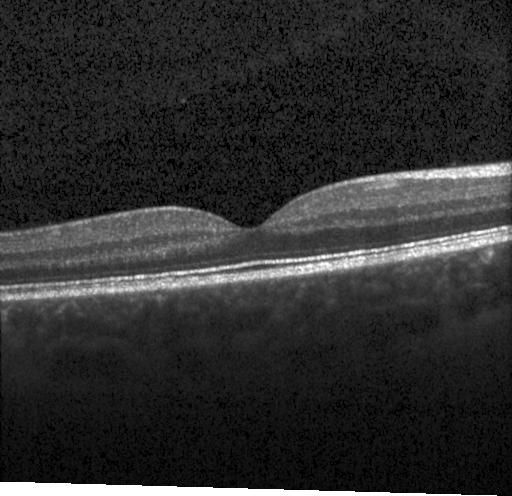

Impression: no evidence of choroidal neovascularization, diabetic macular edema, or drusen.